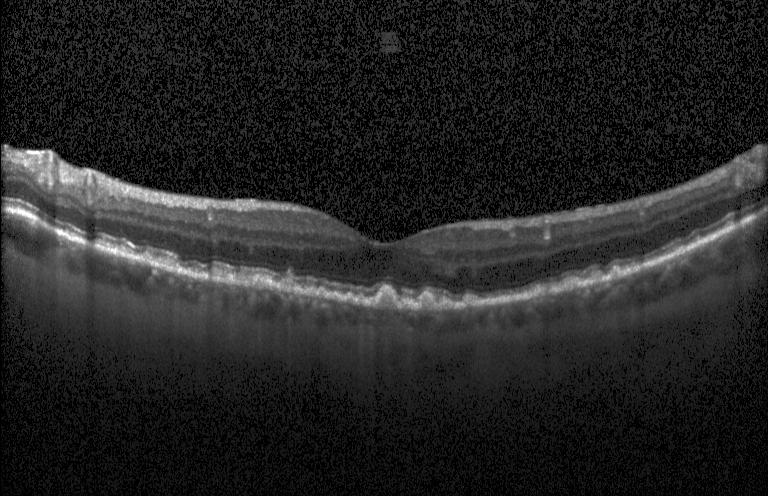

Optical coherence tomography scan, spectral-domain OCT — OCT finding: drusen.